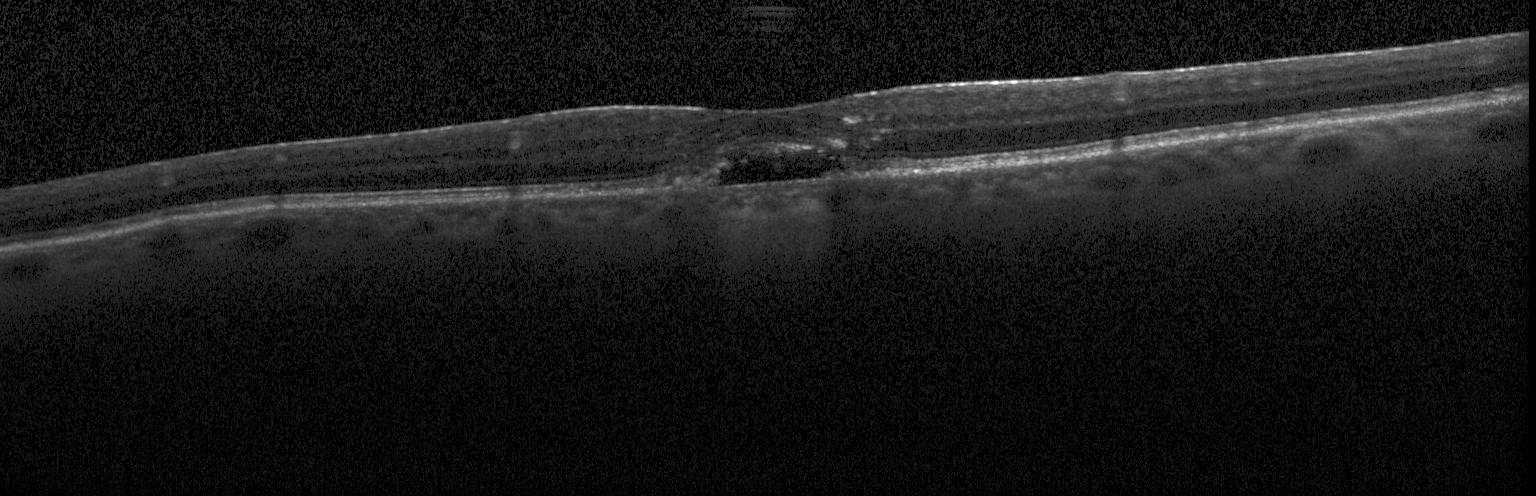
Macular OCT: a choroidal neovascular membrane.